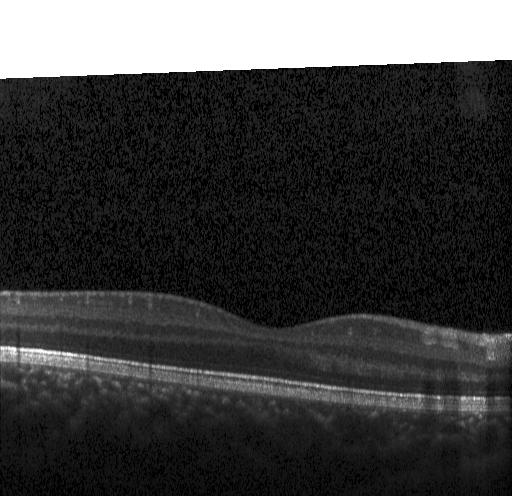

Macular OCT: neither CNV, DME, nor drusen.